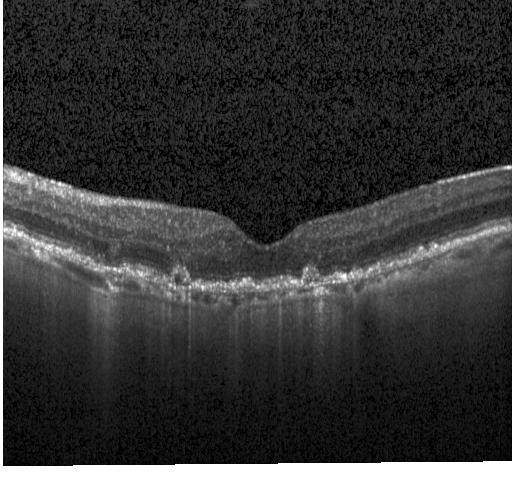
Dx: a choroidal neovascular membrane.